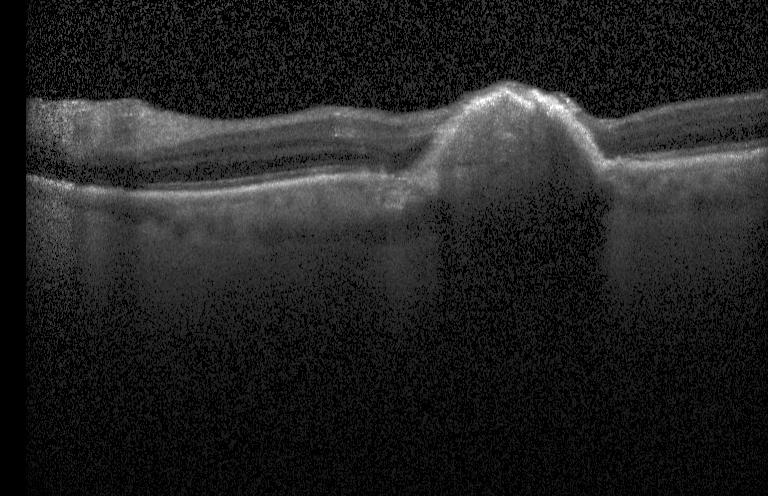
Diagnosis: choroidal neovascularization.